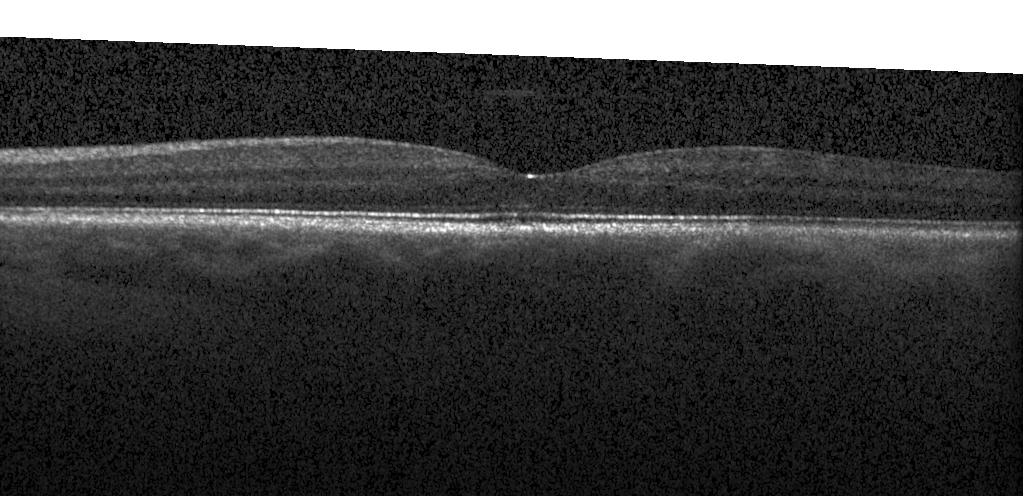 Optical coherence tomography B-scan, acquired on a Heidelberg Spectralis. Impression: no evidence of choroidal neovascularization, diabetic macular edema, or drusen.